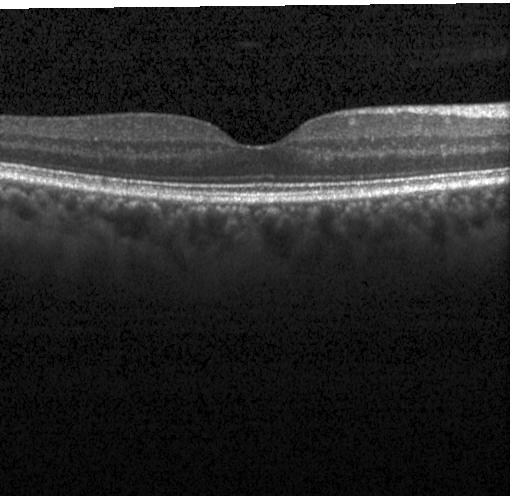
Heidelberg Spectralis; OCT B-scan — Macular OCT: neither choroidal neovascularization, diabetic macular edema, nor drusen.